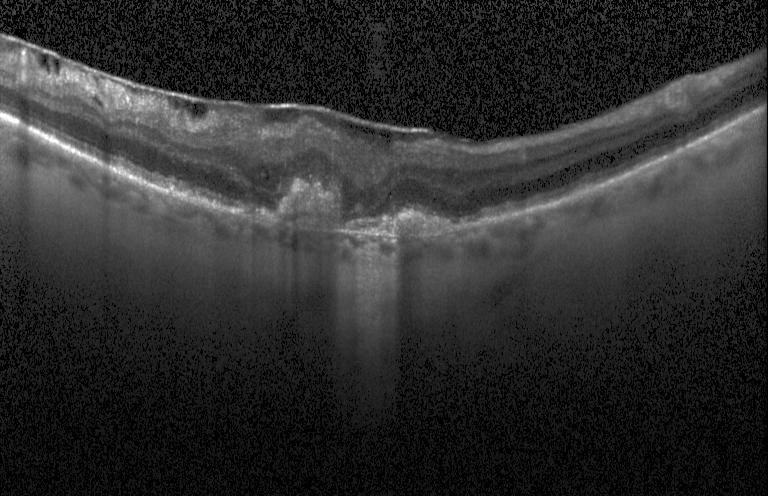
OCT B-scan; Heidelberg Spectralis OCT system; SD-OCT — Assessment: a choroidal neovascular membrane.